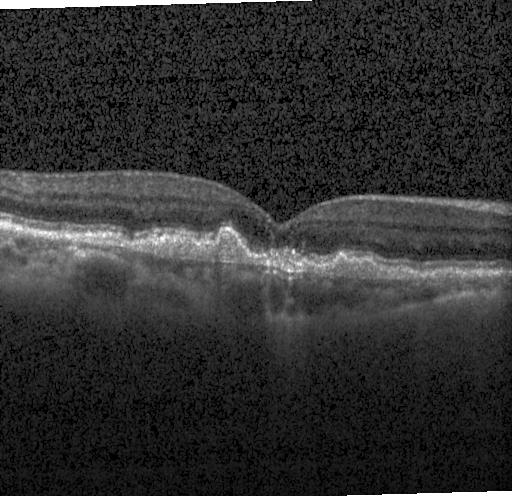 Instrument: Heidelberg Spectralis · fovea-centered · SD-OCT · OCT line scan — Finding: a choroidal neovascular membrane.